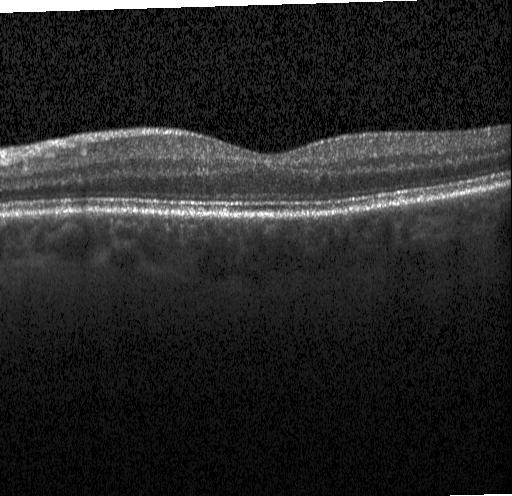 Macular scan, OCT B-scan, spectral-domain OCT
Impression: no evidence of CNV, DME, or drusen.